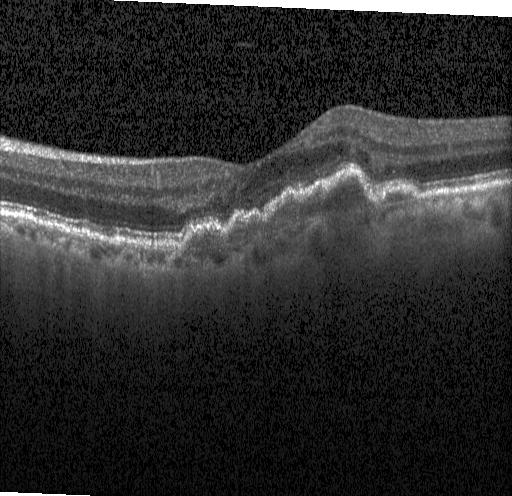 Optical coherence tomography scan, instrument: Heidelberg Spectralis, spectral-domain OCT.
Diagnosis: choroidal neovascularization.